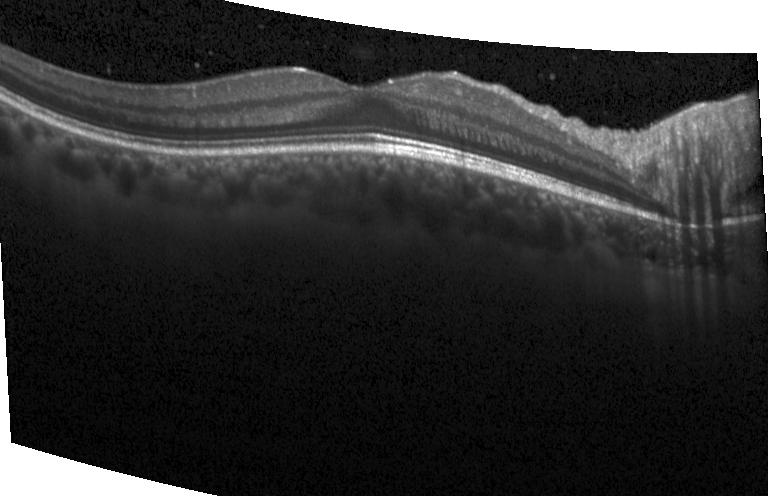 OCT B-scan.
Finding: neither choroidal neovascularization, diabetic macular edema, nor drusen.